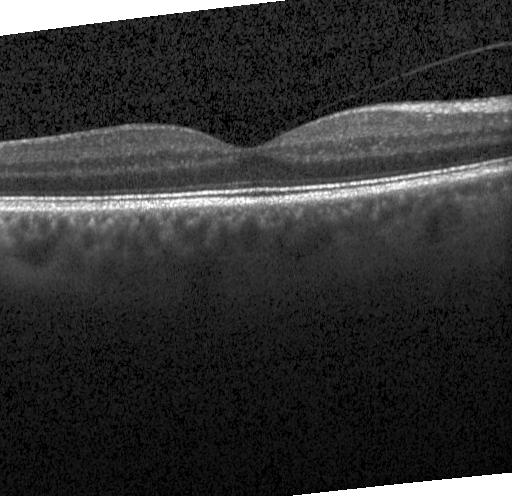 Optical coherence tomography scan — Impression: no choroidal neovascularization, no diabetic macular edema, and no drusen.